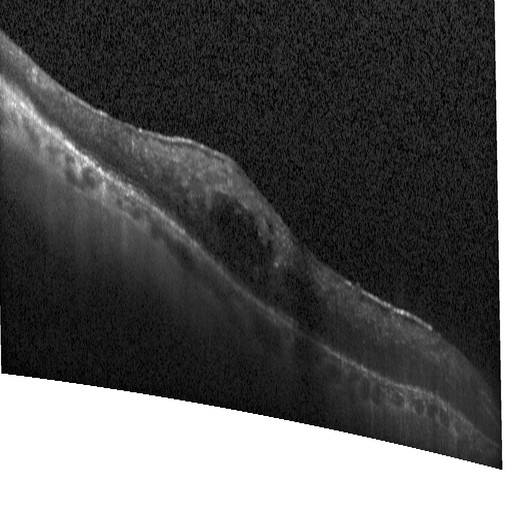

Retinal OCT cross-section; centered on the fovea.
Diagnosis: diabetic macular edema (DME).